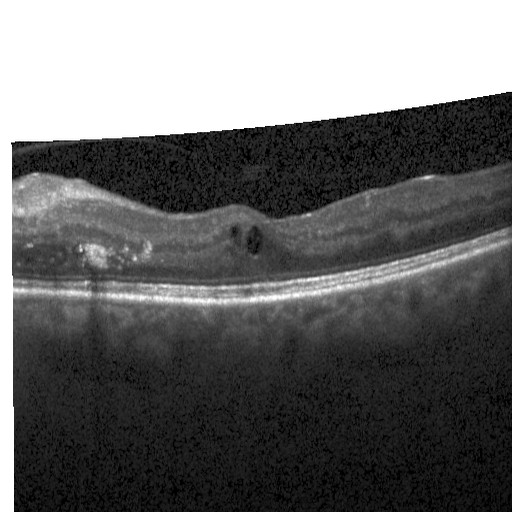
Assessment: diabetic macular edema (DME).